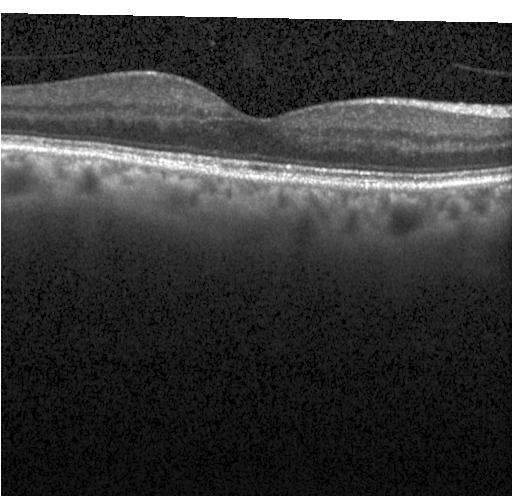
SD-OCT, retinal OCT cross-section, macular scan.
Diagnosis: neither choroidal neovascularization, diabetic macular edema, nor drusen.